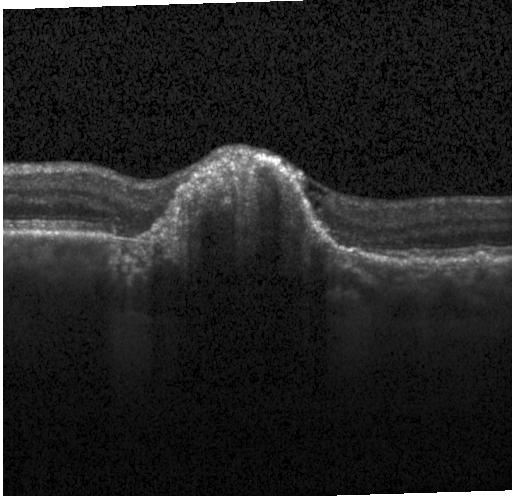
Finding: choroidal neovascularization (CNV).